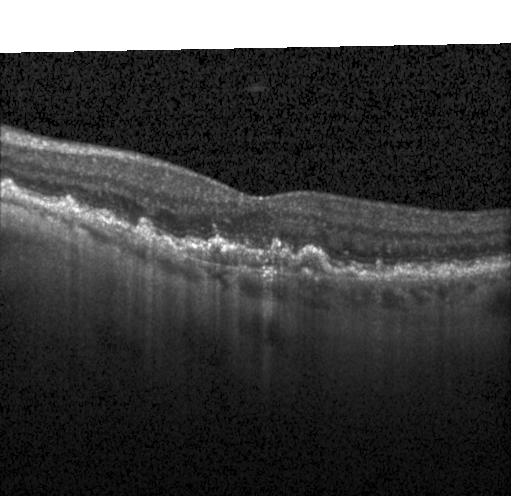
OCT scan showing a choroidal neovascular membrane.